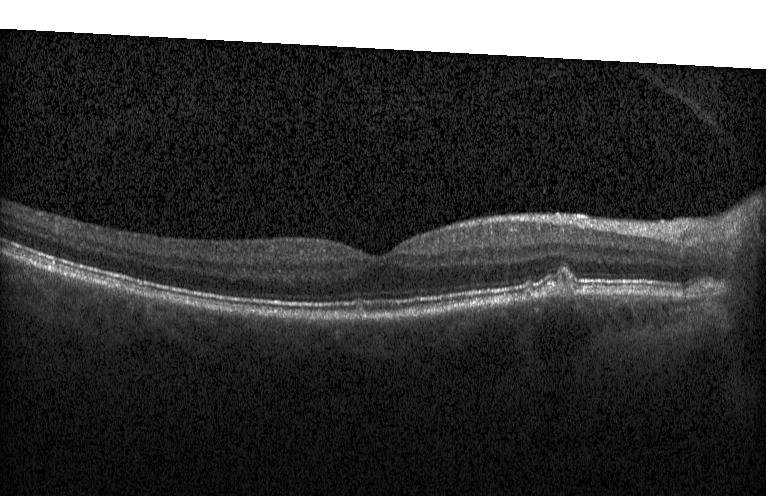

Optical coherence tomography B-scan.
Diagnosis: sub-RPE drusenoid deposits.